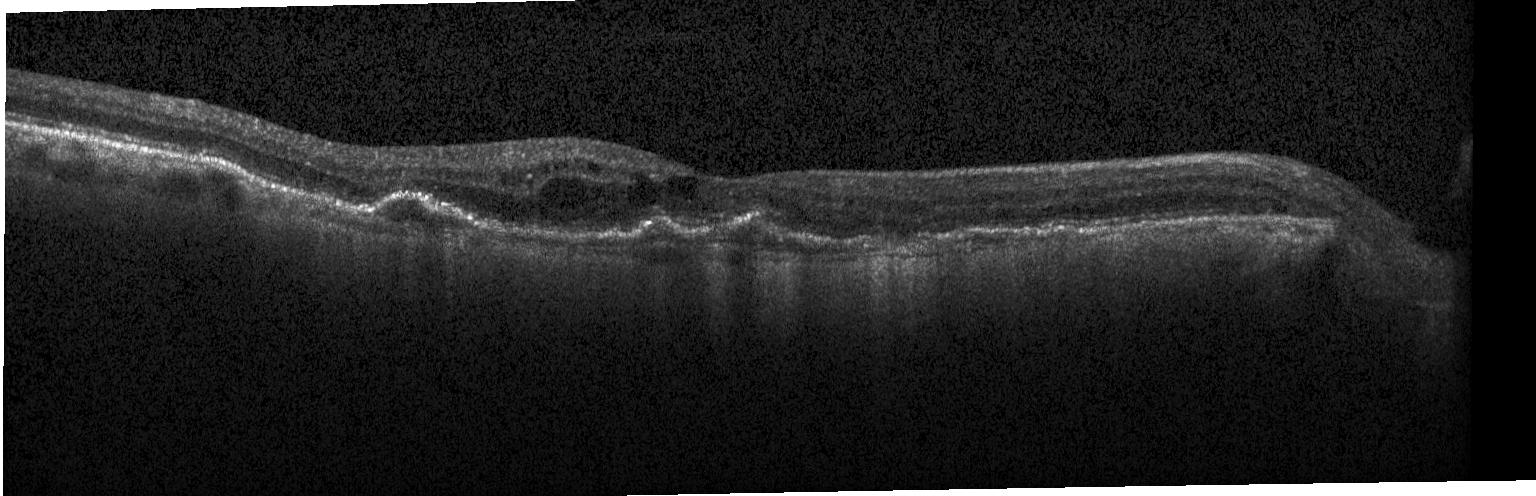

Heidelberg Spectralis · retinal OCT B-scan · SD-OCT.
Assessment: a choroidal neovascular membrane.